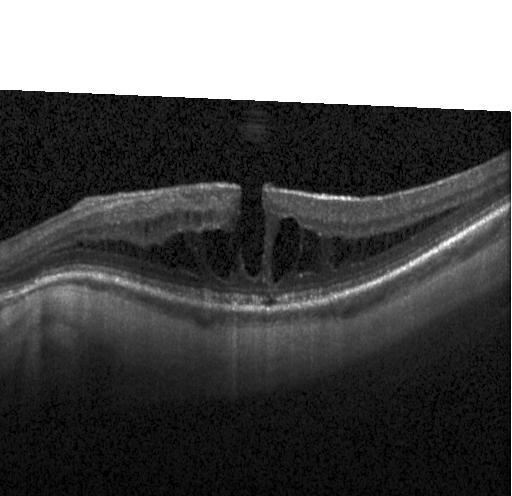

Instrument: Heidelberg Spectralis · retinal OCT B-scan · horizontal scan through the fovea · SD-OCT.
OCT finding: DME.